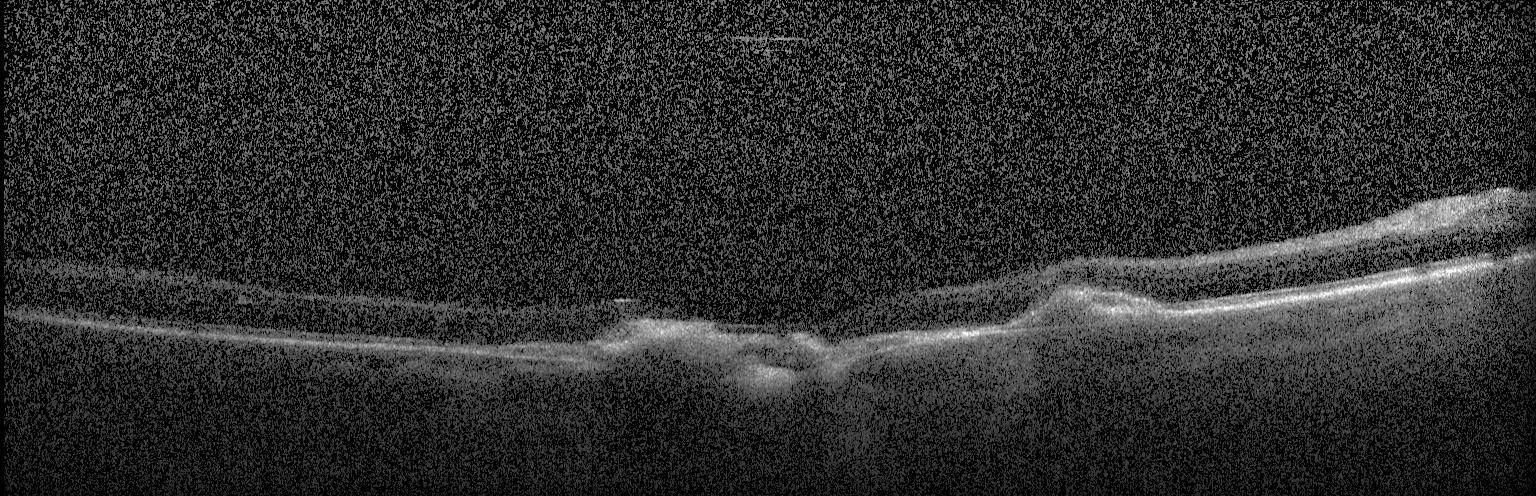 Retinal OCT B-scan — This B-scan demonstrates CNV.